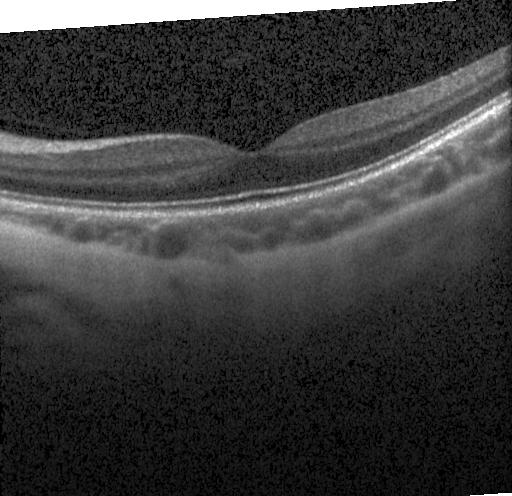

Retinal OCT B-scan, SD-OCT, acquired on a Heidelberg Spectralis, through the macula.
Dx: no choroidal neovascularization, diabetic macular edema, or drusen.